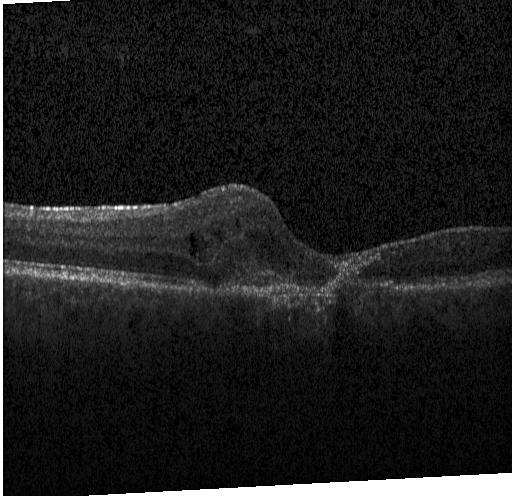
Impression: choroidal neovascularization.